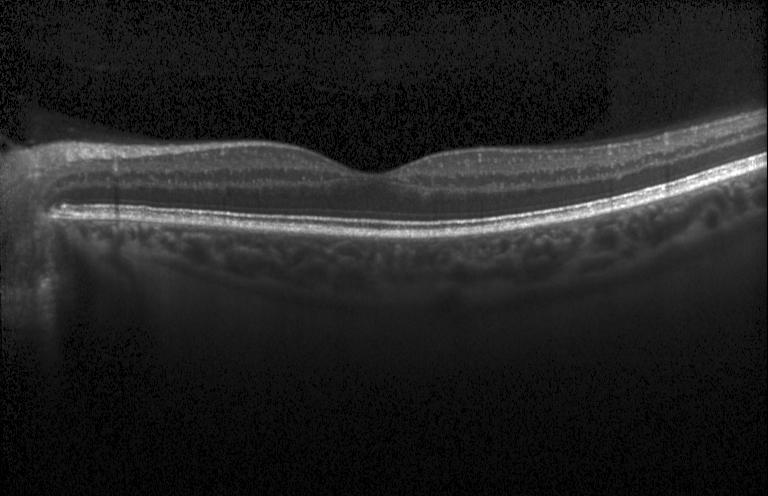 Optical coherence tomography scan. Impression: no choroidal neovascularization, diabetic macular edema, or drusen.